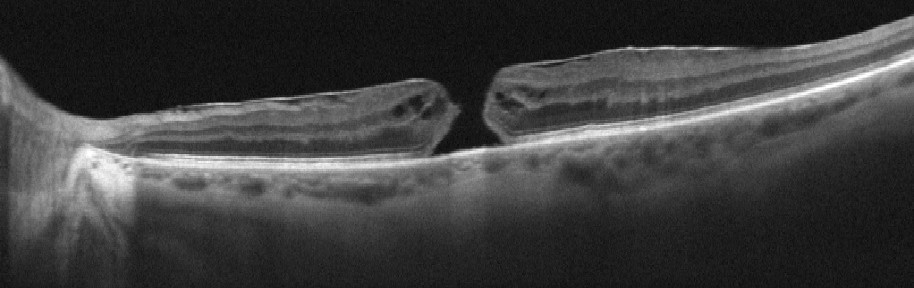 OCT B-scan
Dx: vitreomacular interface disease.